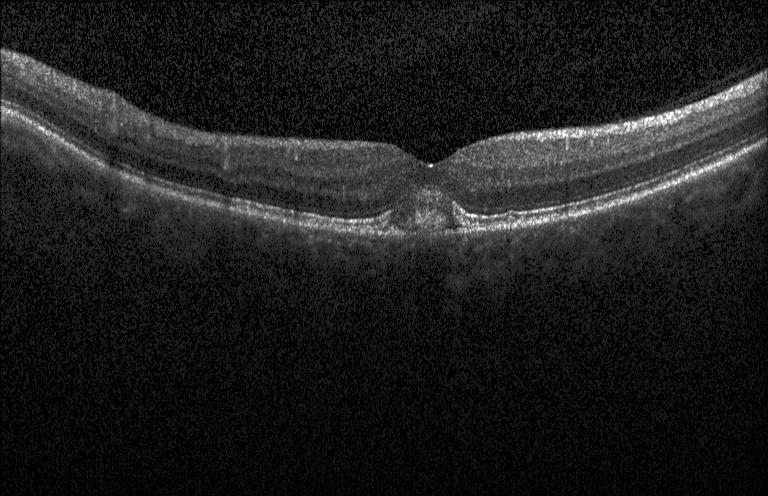
OCT B-scan; spectral-domain optical coherence tomography; macular scan; Heidelberg Spectralis
This B-scan demonstrates choroidal neovascularization (CNV).